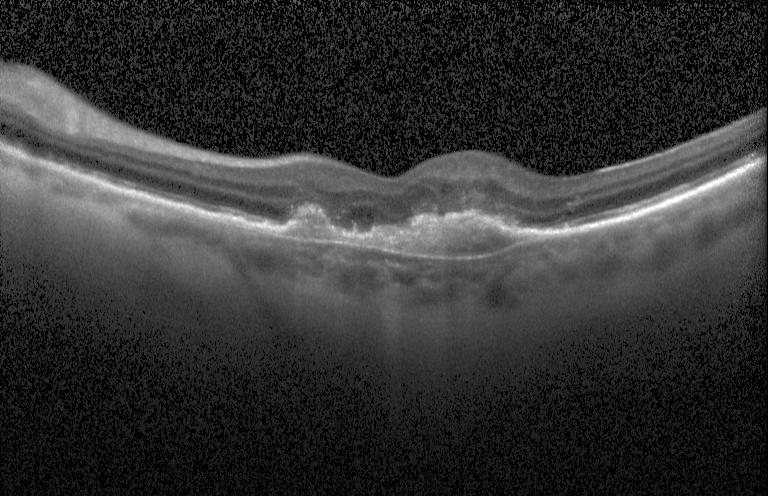

Centered on the fovea · spectral-domain OCT · retinal OCT B-scan
Finding: CNV.